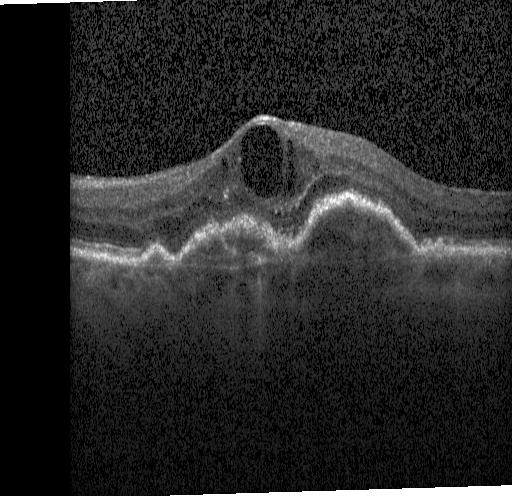 Dx: choroidal neovascularization.